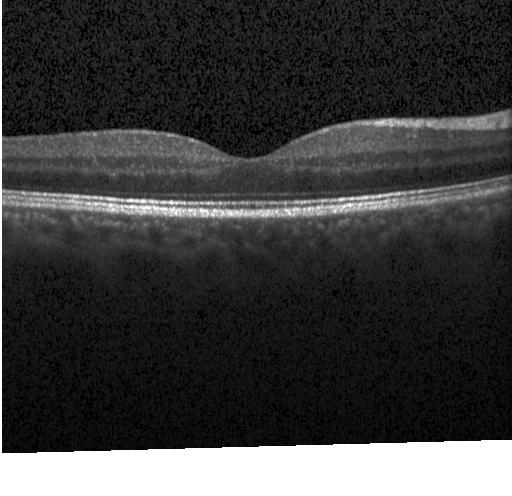 Macular scan · Heidelberg Spectralis OCT system · SD-OCT · OCT B-scan. OCT finding: no choroidal neovascularization, diabetic macular edema, or drusen.